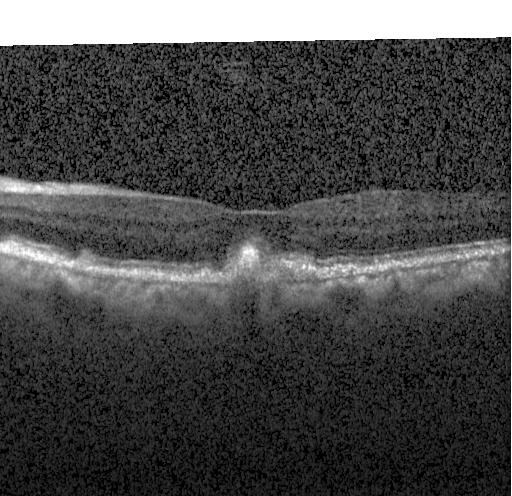

Retinal OCT B-scan
Finding: a choroidal neovascular membrane.